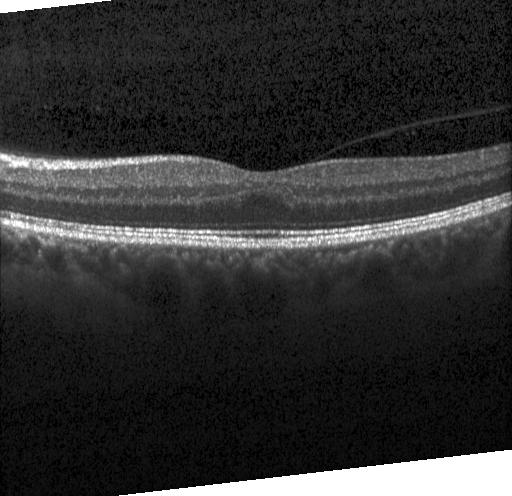 Retinal OCT B-scan, instrument: Heidelberg Spectralis, fovea-centered. This B-scan demonstrates neither choroidal neovascularization, diabetic macular edema, nor drusen.